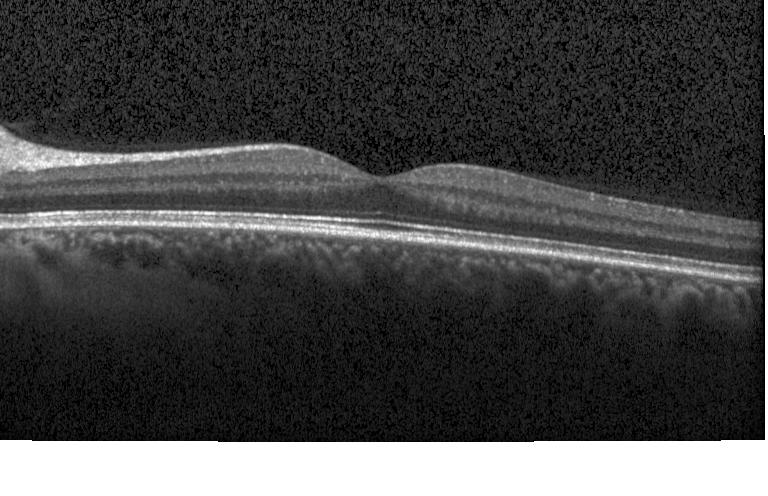

Finding: no evidence of choroidal neovascularization, diabetic macular edema, or drusen.